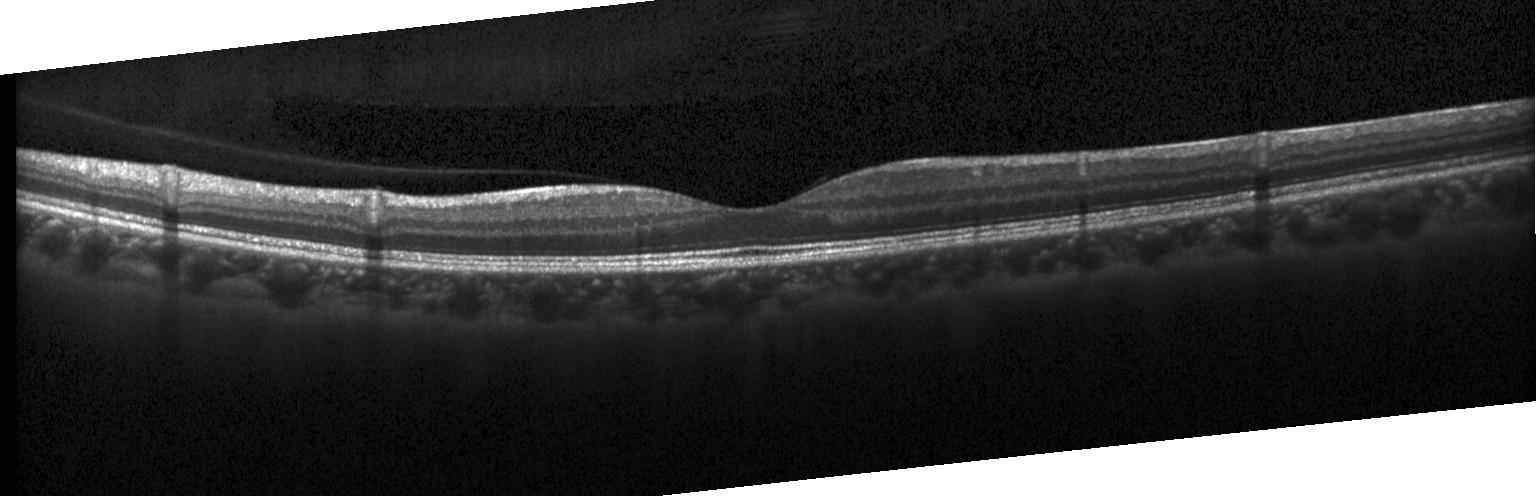

Spectral-domain optical coherence tomography; OCT B-scan; instrument: Heidelberg Spectralis. This B-scan demonstrates no choroidal neovascularization, diabetic macular edema, or drusen.